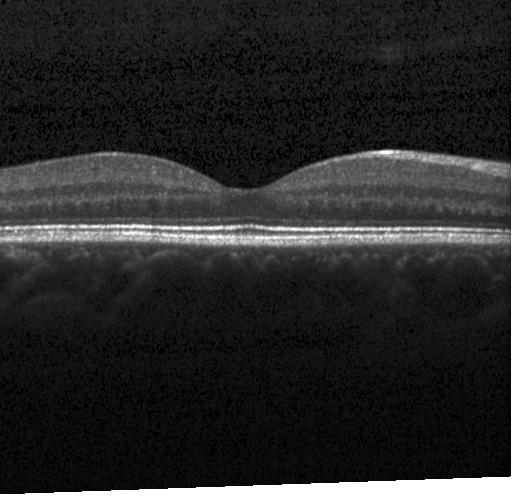
Acquired on a Heidelberg Spectralis. OCT B-scan — Impression: no evidence of choroidal neovascularization, diabetic macular edema, or drusen.